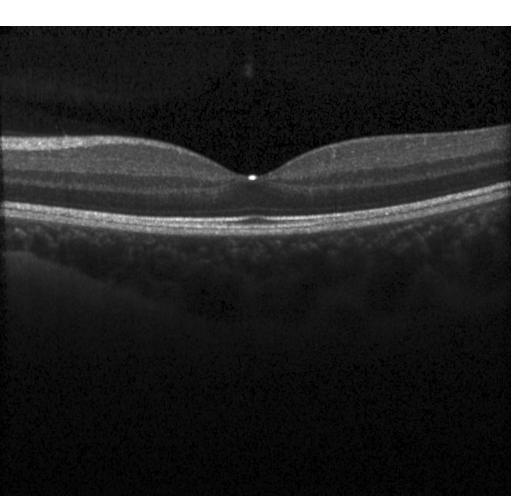

Impression: no evidence of choroidal neovascularization, diabetic macular edema, or drusen.